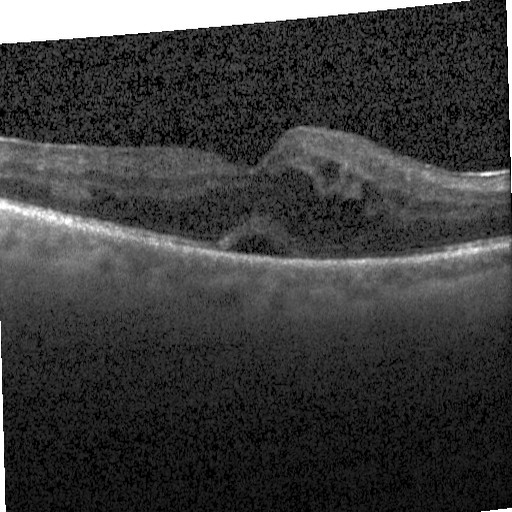

Impression: DME.